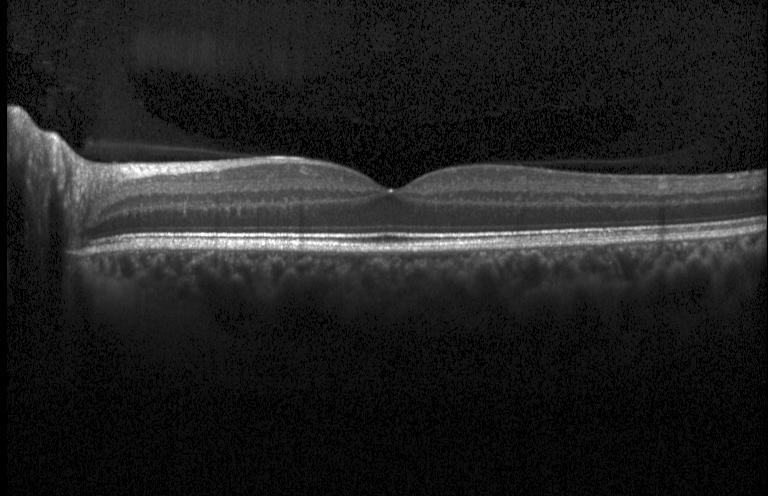
OCT B-scan; acquired on a Heidelberg Spectralis; SD-OCT
Dx: neither choroidal neovascularization, diabetic macular edema, nor drusen.